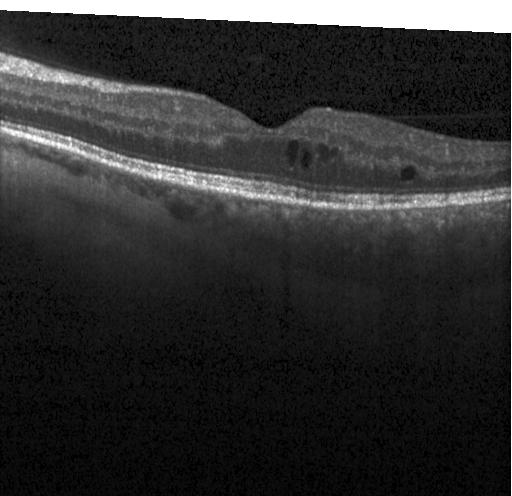
Acquired on a Heidelberg Spectralis · centered on the fovea · optical coherence tomography B-scan · spectral-domain optical coherence tomography. Impression: diabetic macular edema (DME).